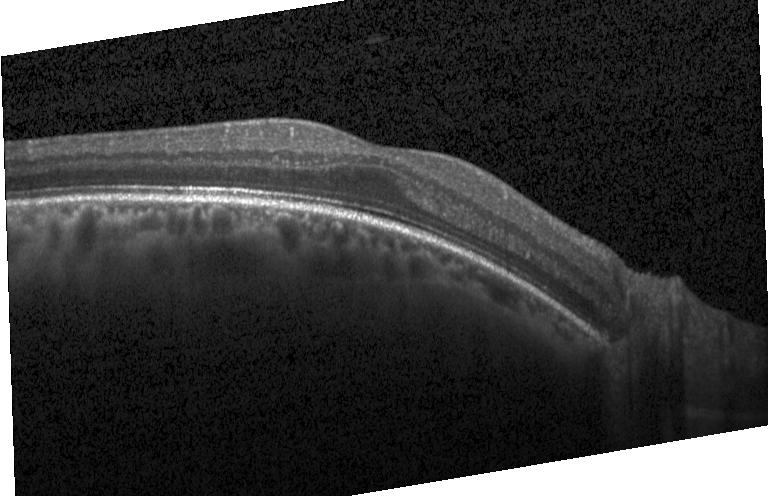

OCT line scan; horizontal scan through the fovea; Heidelberg Spectralis OCT system; spectral-domain optical coherence tomography.
No choroidal neovascularization, no diabetic macular edema, and no drusen.